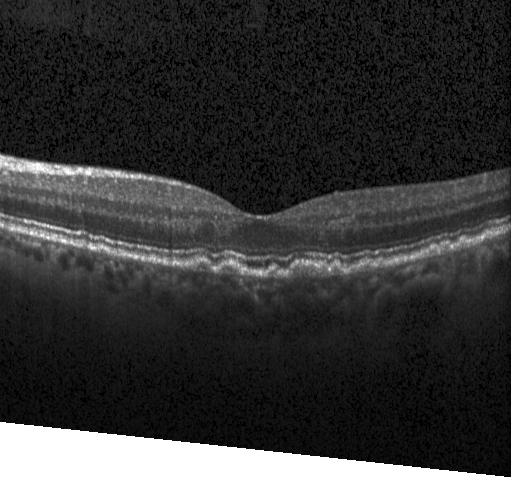
Finding: sub-RPE drusenoid deposits.